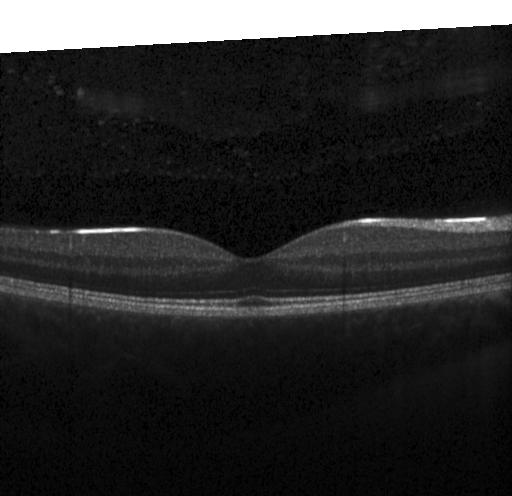
OCT B-scan — Diagnosis: neither choroidal neovascularization, diabetic macular edema, nor drusen.